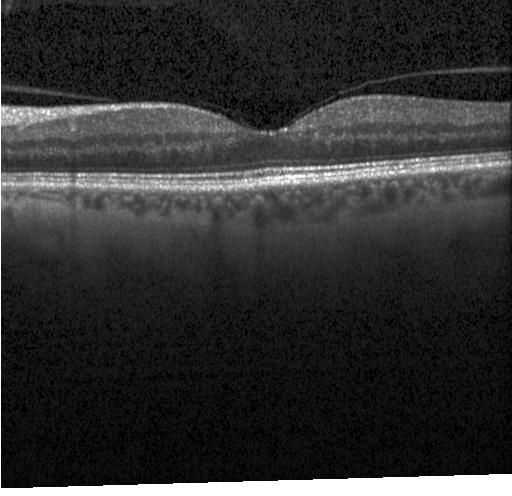 Impression: no choroidal neovascularization, no diabetic macular edema, and no drusen.